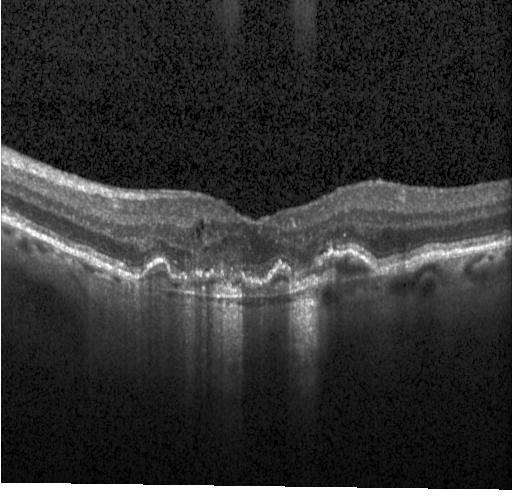

The scan shows a choroidal neovascular membrane.